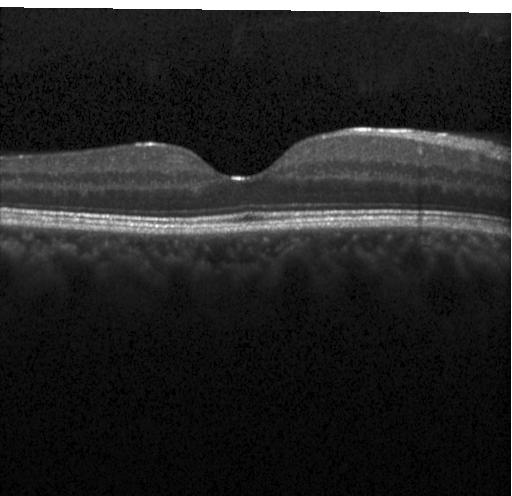
No CNV, no DME, and no drusen.